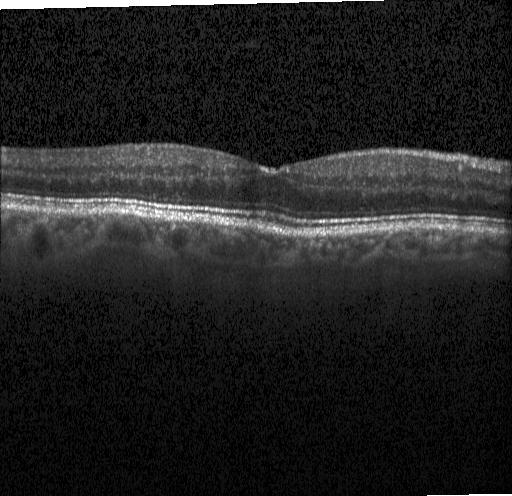
Retinal OCT B-scan, spectral-domain optical coherence tomography, instrument: Heidelberg Spectralis.
Impression: neither choroidal neovascularization, diabetic macular edema, nor drusen.